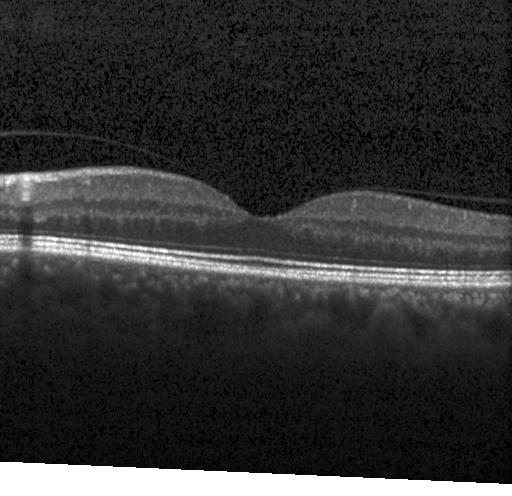 OCT B-scan. Assessment: no CNV, DME, or drusen.